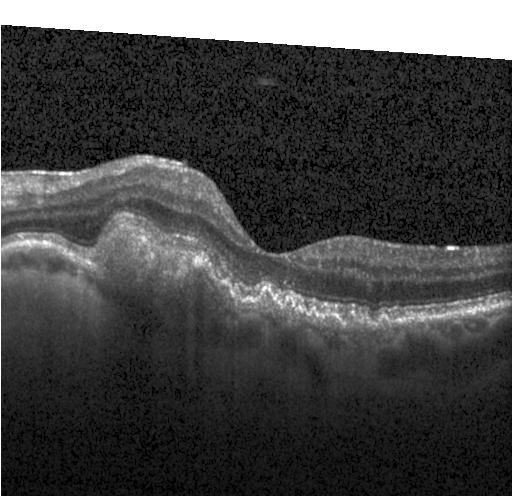 Through the macula · retinal OCT cross-section · spectral-domain optical coherence tomography
Macular OCT: a choroidal neovascular membrane.